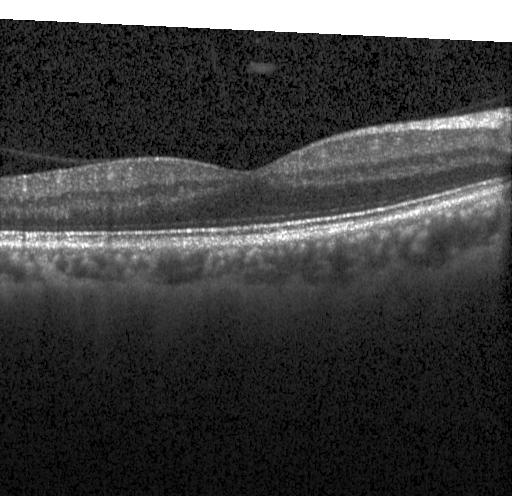

Dx: no choroidal neovascularization, no diabetic macular edema, and no drusen.